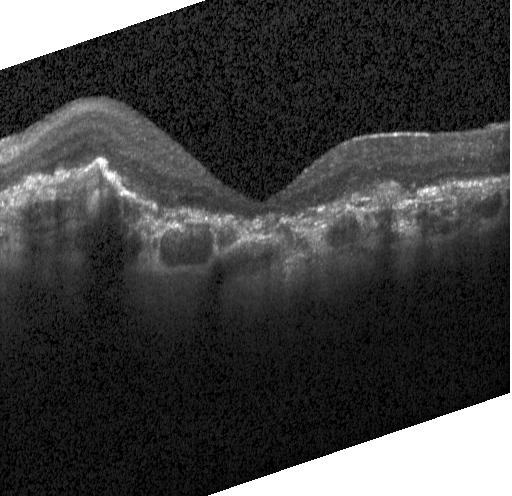 Impression: CNV.